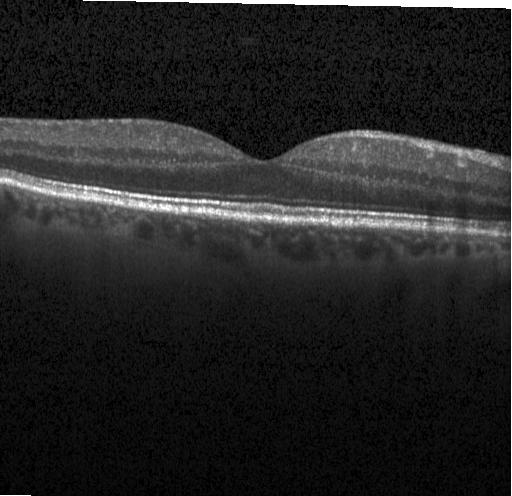 Diagnosis: no choroidal neovascularization, diabetic macular edema, or drusen.